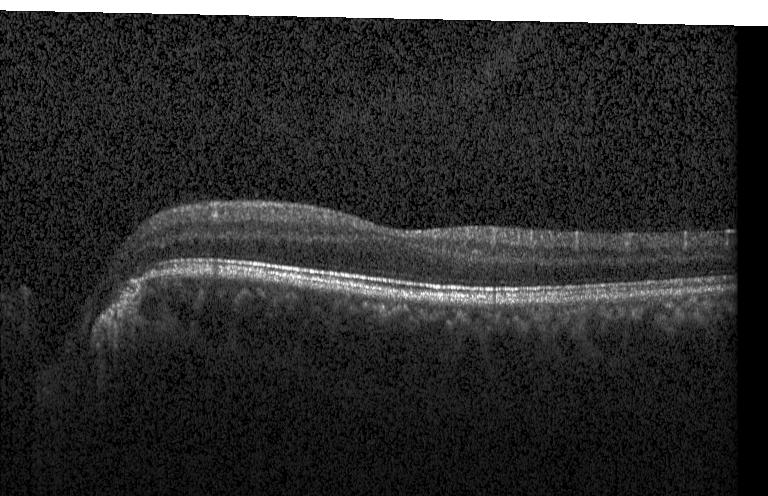
OCT scan showing no choroidal neovascularization, diabetic macular edema, or drusen.